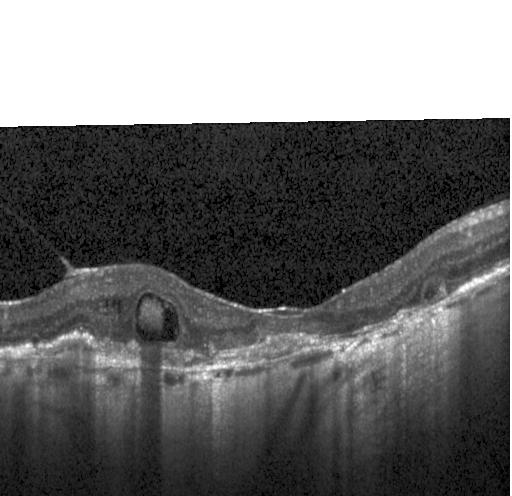
Optical coherence tomography B-scan; Heidelberg Spectralis OCT system.
OCT finding: a choroidal neovascular membrane.